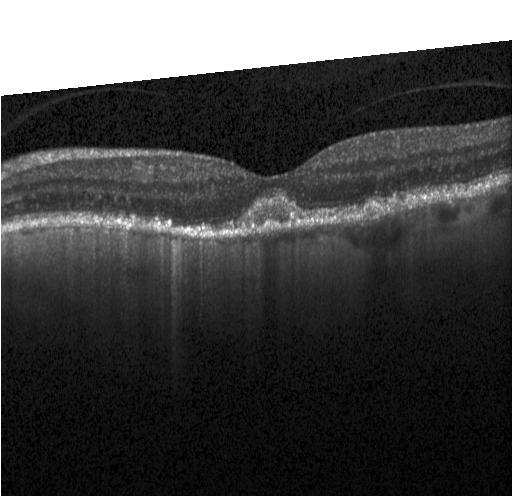

Finding: multiple drusen.